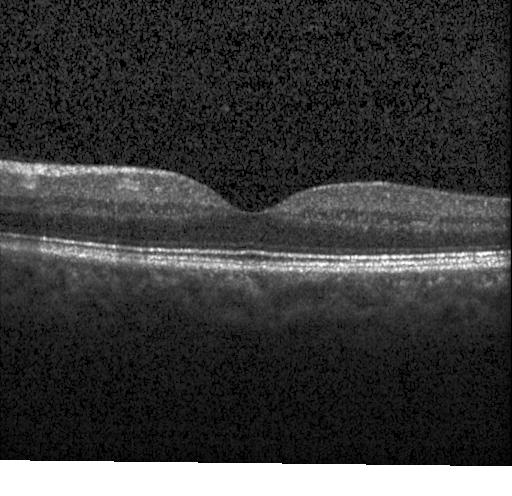
Acquired on a Heidelberg Spectralis · SD-OCT · OCT line scan
No choroidal neovascularization, no diabetic macular edema, and no drusen.